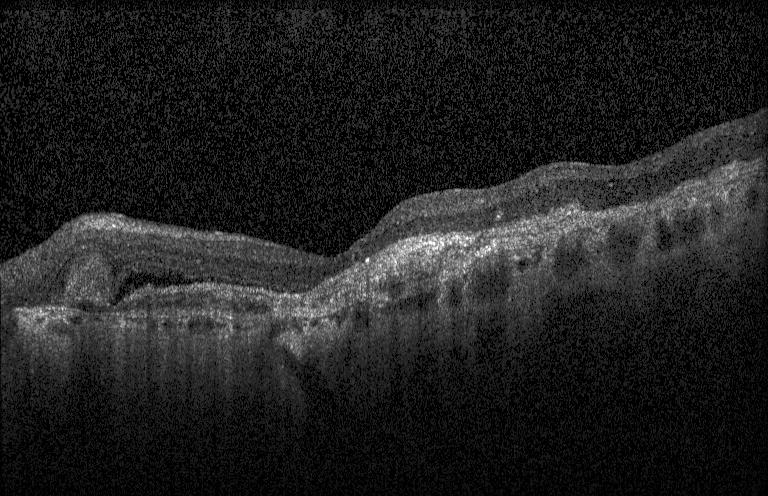 Finding: a choroidal neovascular membrane.